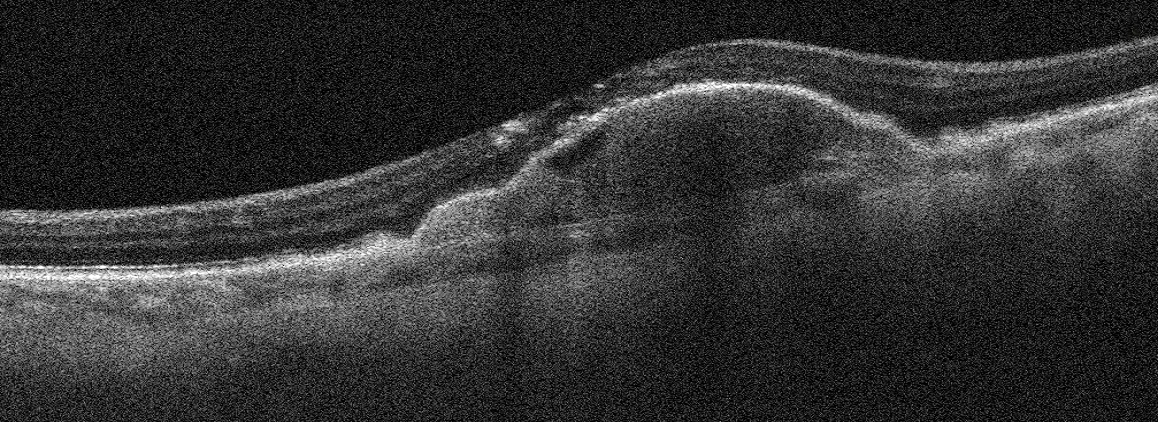
Optical coherence tomography B-scan; right eye
This B-scan demonstrates age-related macular degeneration (AMD).